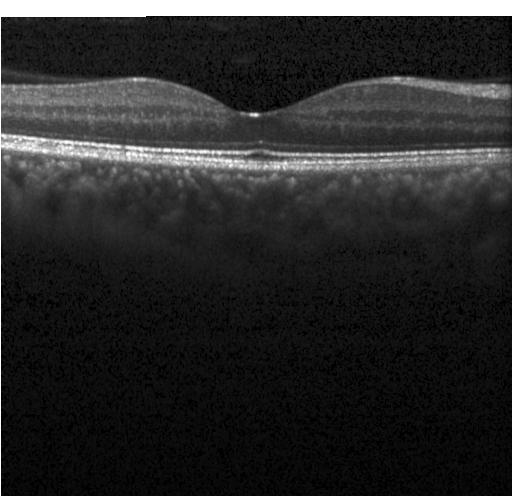 The scan shows no CNV, DME, or drusen.